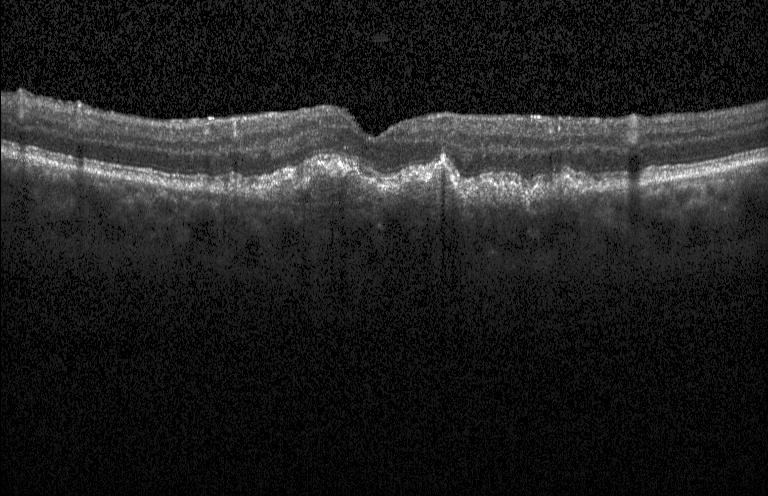

Acquired on a Heidelberg Spectralis · spectral-domain optical coherence tomography · fovea-centered · retinal OCT B-scan.
The scan shows choroidal neovascularization (CNV).